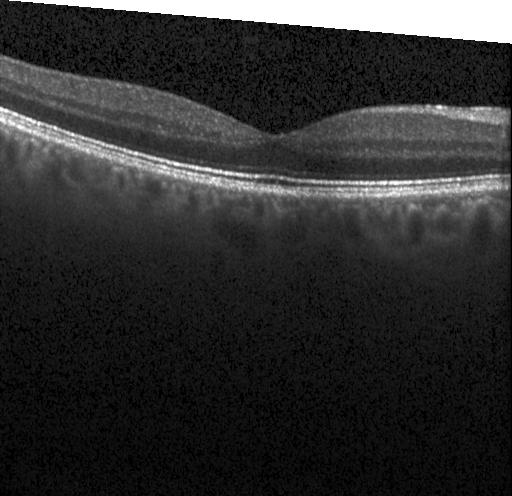
Optical coherence tomography scan, SD-OCT
Diagnosis: no choroidal neovascularization, no diabetic macular edema, and no drusen.